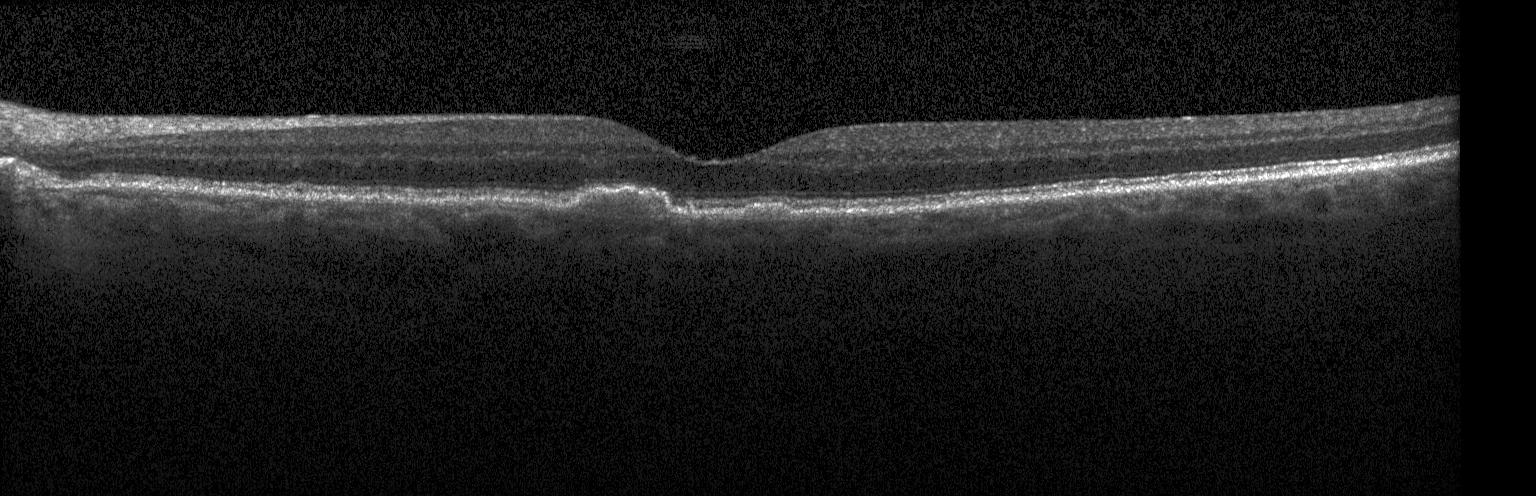

Assessment: drusen.